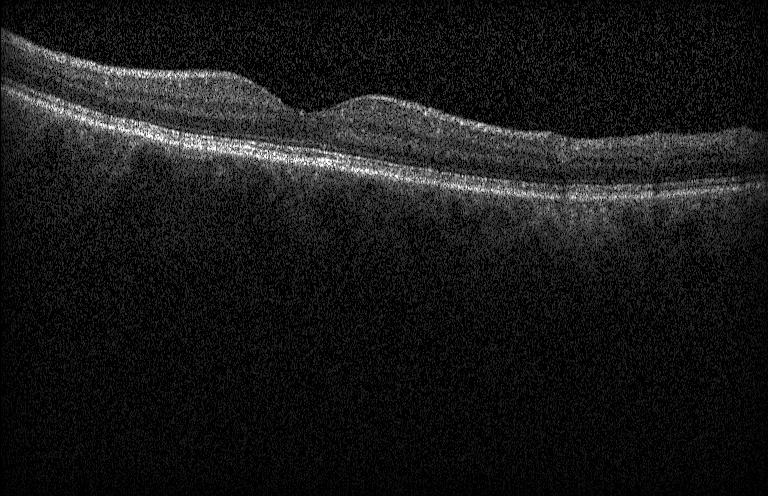

Optical coherence tomography B-scan
Assessment: no choroidal neovascularization, no diabetic macular edema, and no drusen.